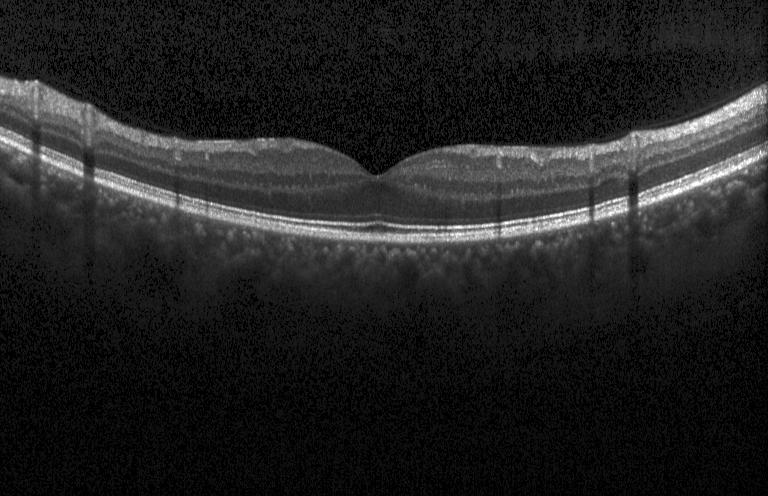 Optical coherence tomography scan. Through the macula
Dx: neither choroidal neovascularization, diabetic macular edema, nor drusen.